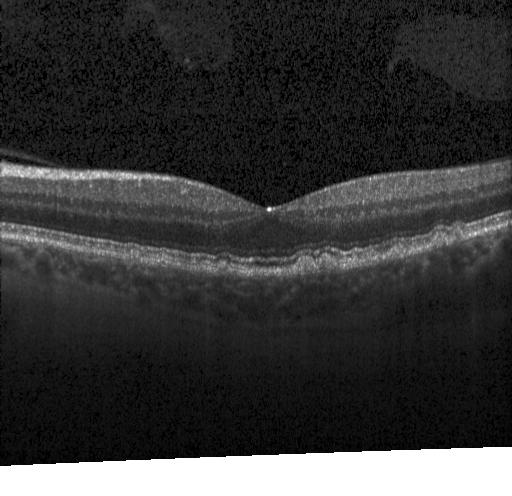

Finding: sub-RPE drusenoid deposits.